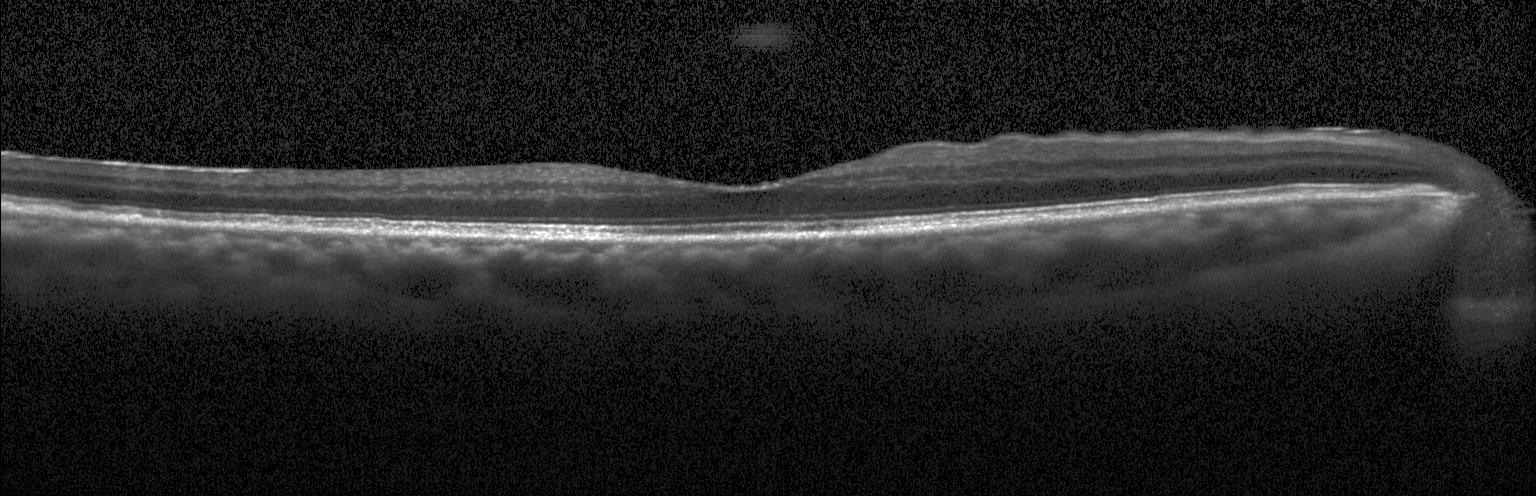 This B-scan demonstrates neither choroidal neovascularization, diabetic macular edema, nor drusen.